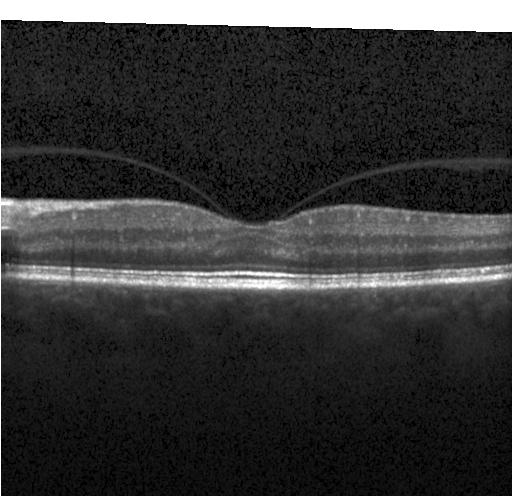 Optical coherence tomography scan, spectral-domain optical coherence tomography. This B-scan demonstrates no evidence of choroidal neovascularization, diabetic macular edema, or drusen.